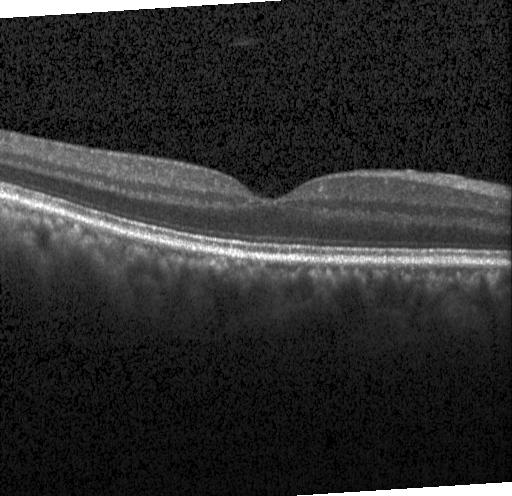
Fovea-centered · OCT B-scan · Heidelberg Spectralis OCT system · SD-OCT
OCT finding: no evidence of choroidal neovascularization, diabetic macular edema, or drusen.